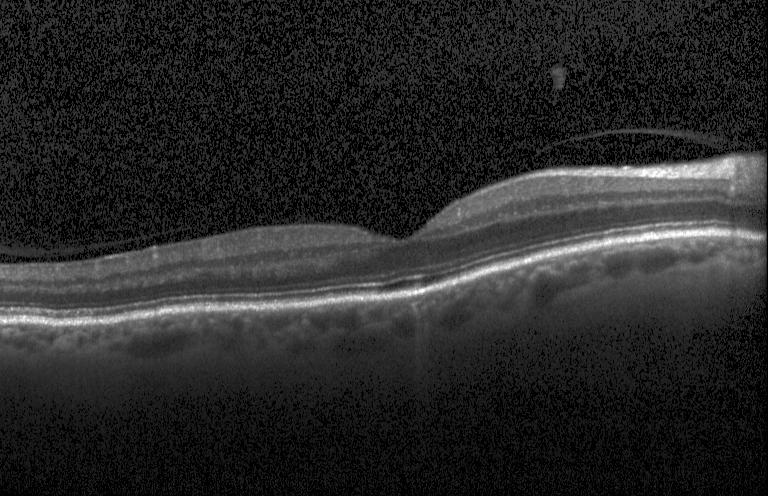

Heidelberg Spectralis; centered on the fovea; spectral-domain OCT; optical coherence tomography scan — Neither choroidal neovascularization, diabetic macular edema, nor drusen.